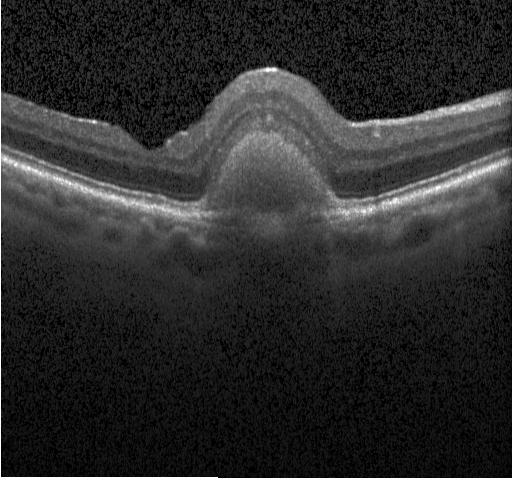
Macular scan · spectral-domain OCT · retinal OCT cross-section. Finding: a choroidal neovascular membrane.